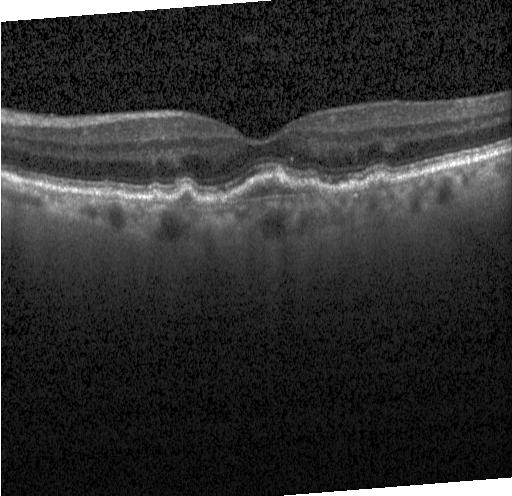 Spectral-domain optical coherence tomography. Acquired on a Heidelberg Spectralis. Retinal OCT cross-section — Finding: a choroidal neovascular membrane.